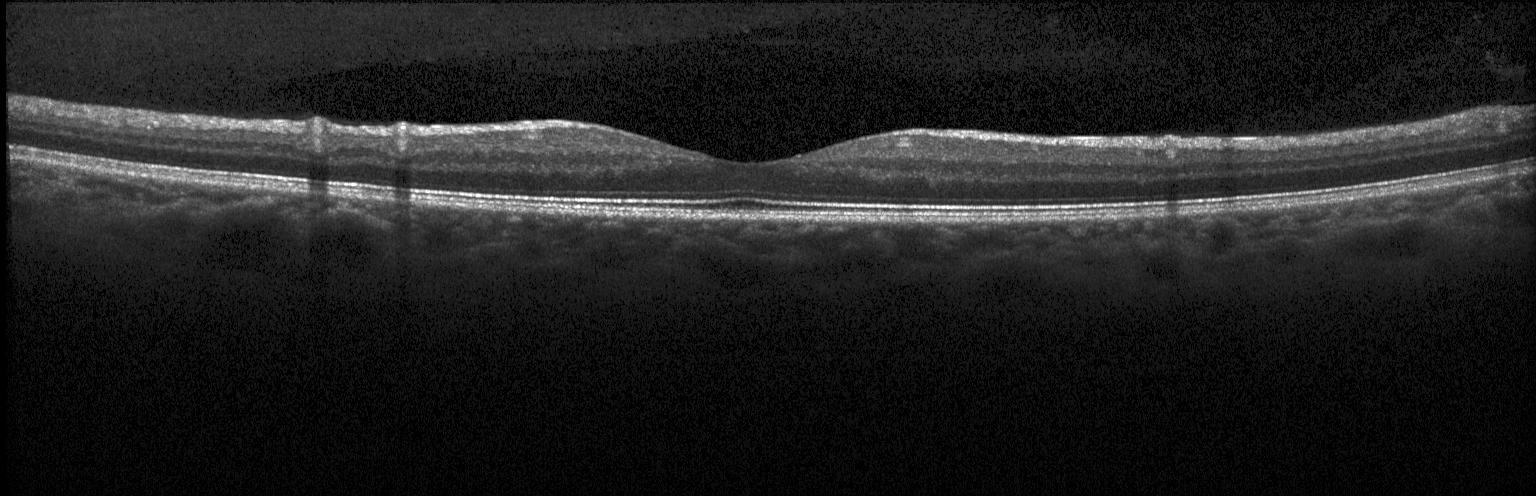 Heidelberg Spectralis OCT system · macular scan · optical coherence tomography B-scan
Finding: no choroidal neovascularization, diabetic macular edema, or drusen.